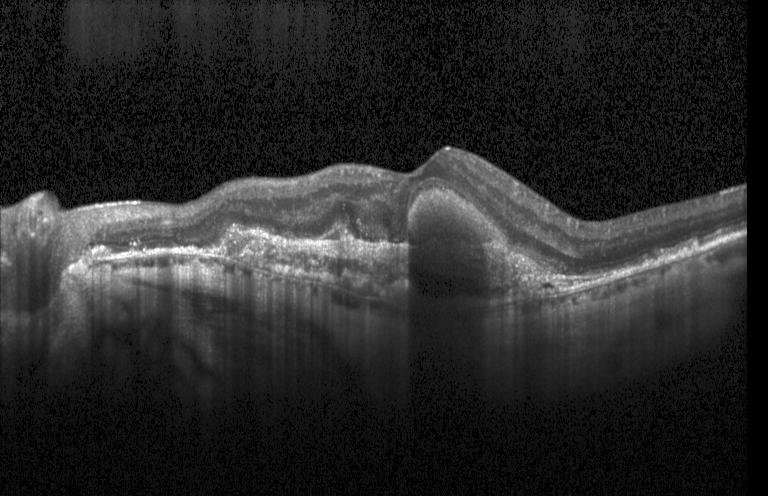

Heidelberg Spectralis OCT system · optical coherence tomography B-scan
Dx: choroidal neovascularization (CNV).